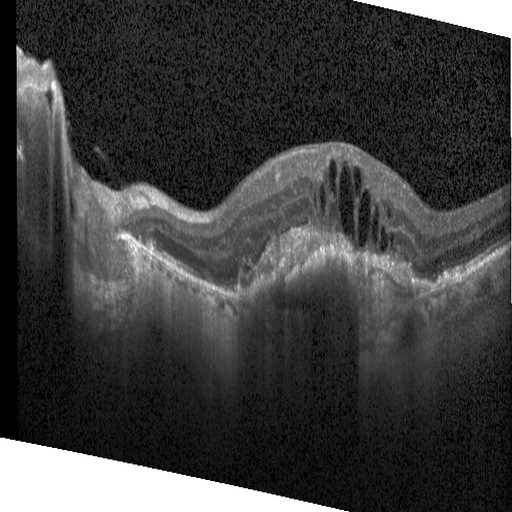
OCT B-scan
Impression: DME.